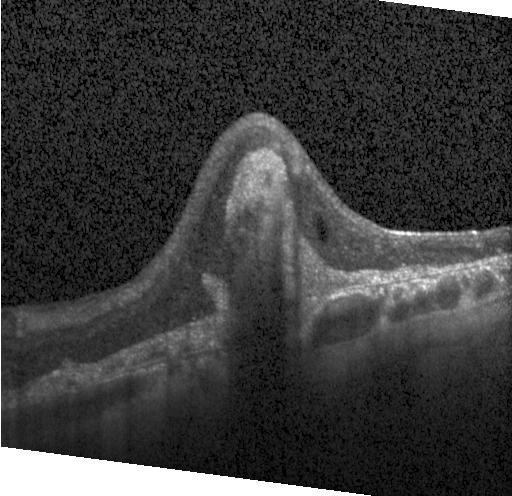

Retinal OCT cross-section showing a choroidal neovascular membrane.